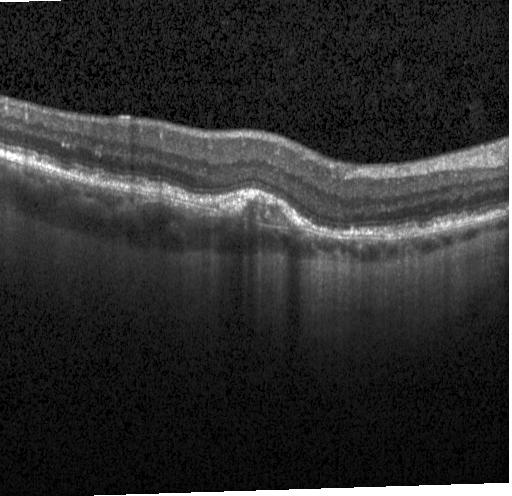 The scan shows a choroidal neovascular membrane.